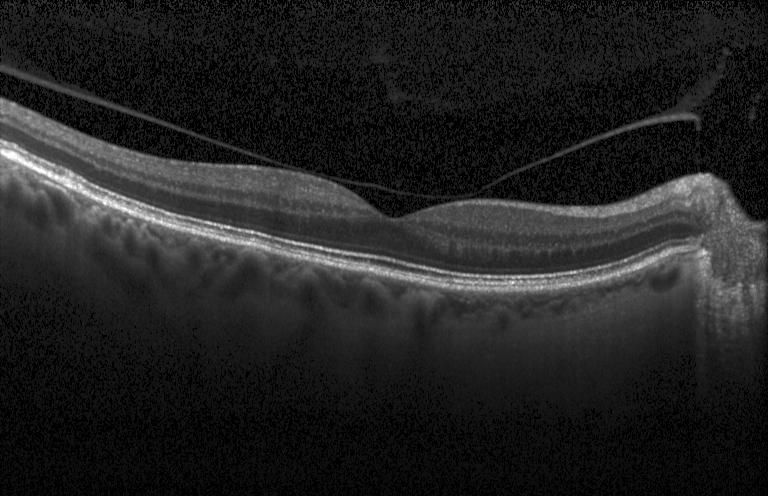 Acquired on a Heidelberg Spectralis; retinal OCT cross-section; horizontal scan through the fovea. OCT finding: no choroidal neovascularization, no diabetic macular edema, and no drusen.